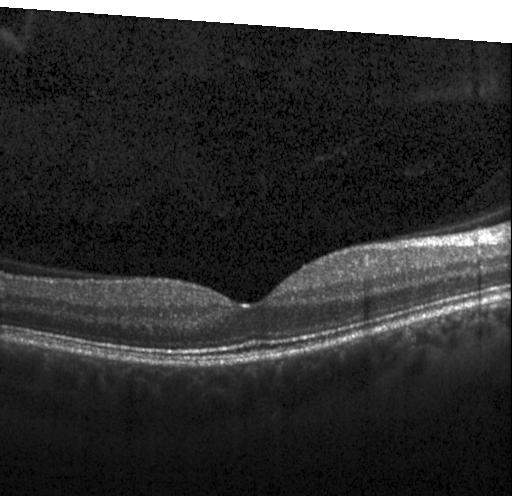
Retinal OCT cross-section.
Impression: no evidence of choroidal neovascularization, diabetic macular edema, or drusen.